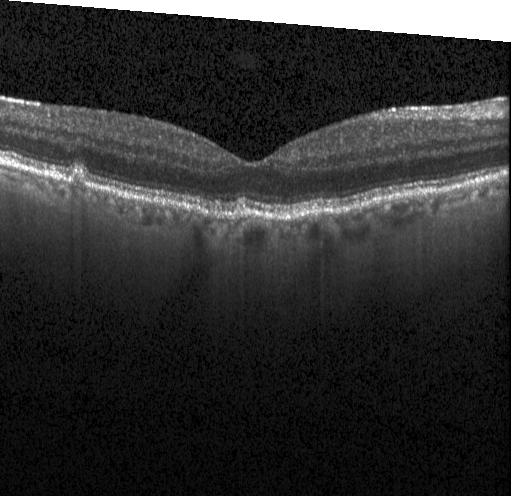

OCT line scan; acquired on a Heidelberg Spectralis; fovea-centered. Impression: multiple drusen.